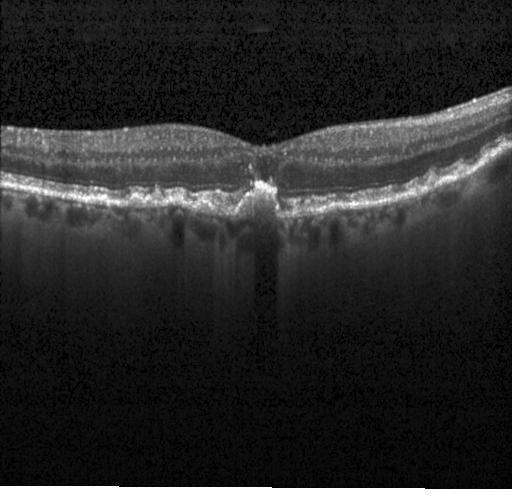
OCT B-scan, centered on the fovea, SD-OCT. Diagnosis: drusen.